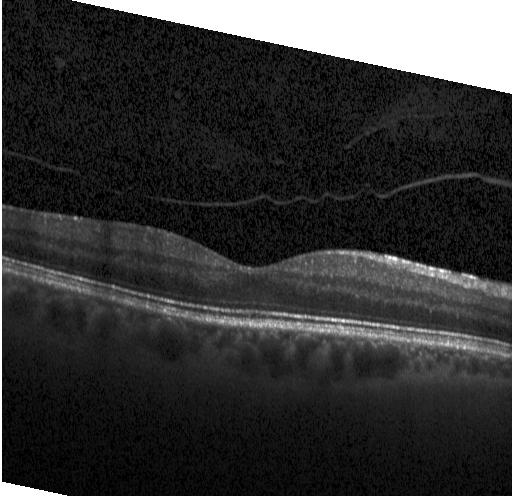 Spectral-domain OCT; optical coherence tomography scan; Heidelberg Spectralis
Assessment: no CNV, no DME, and no drusen.